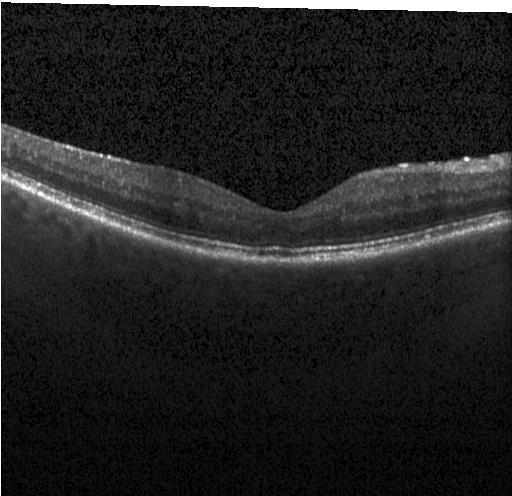

Heidelberg Spectralis OCT system · spectral-domain OCT · macular scan · optical coherence tomography scan
Diagnosis: no CNV, no DME, and no drusen.